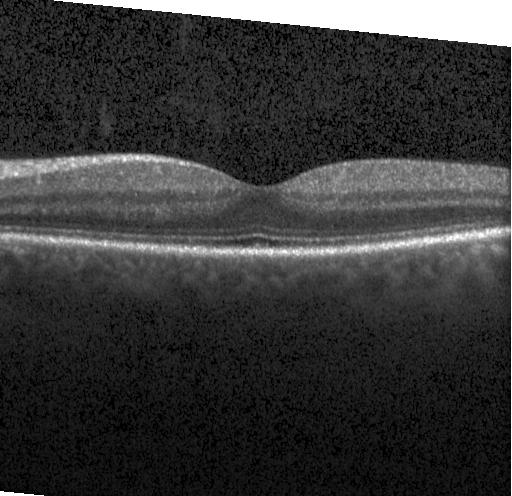

Macular OCT demonstrating no choroidal neovascularization, no diabetic macular edema, and no drusen.